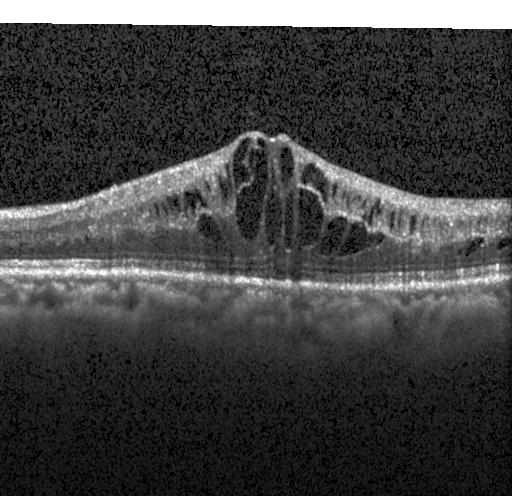
OCT scan showing diabetic macular edema (DME).